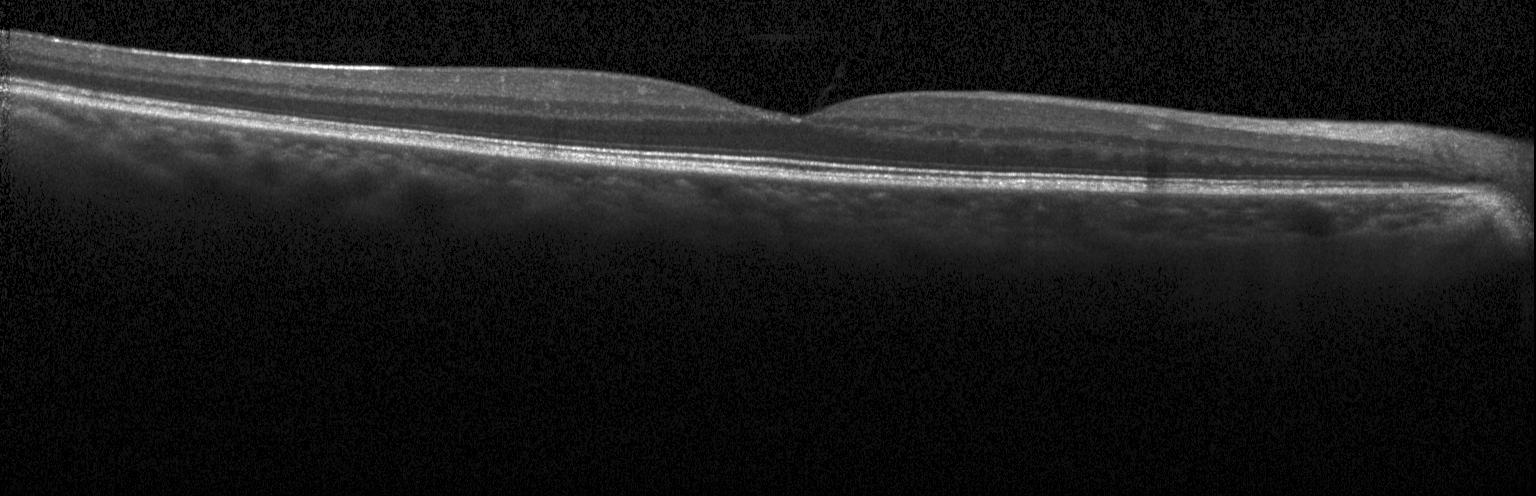

Heidelberg Spectralis; optical coherence tomography B-scan. Finding: no CNV, no DME, and no drusen.